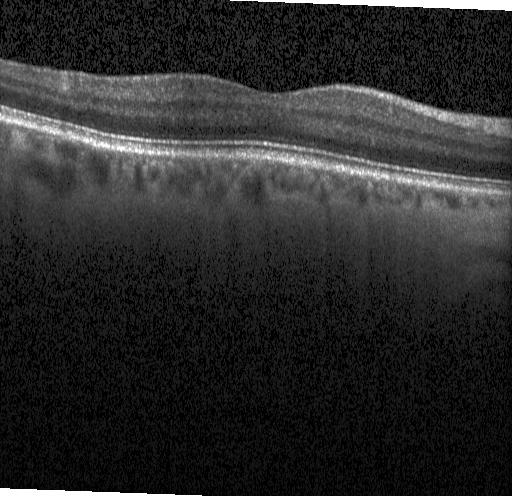

No evidence of choroidal neovascularization, diabetic macular edema, or drusen.